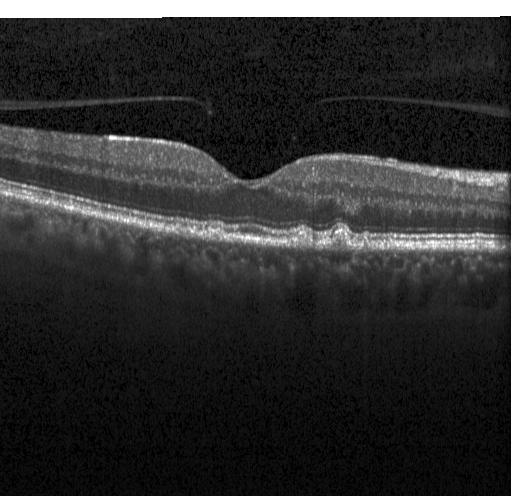 OCT B-scan showing multiple drusen.